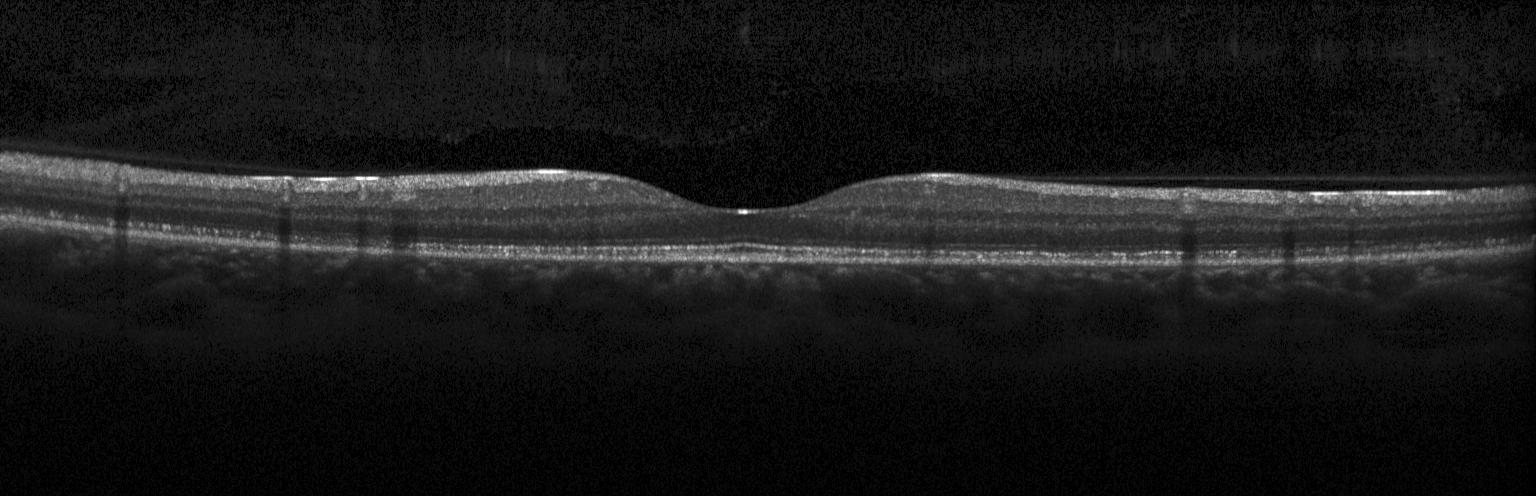

Optical coherence tomography scan
OCT finding: no choroidal neovascularization, no diabetic macular edema, and no drusen.